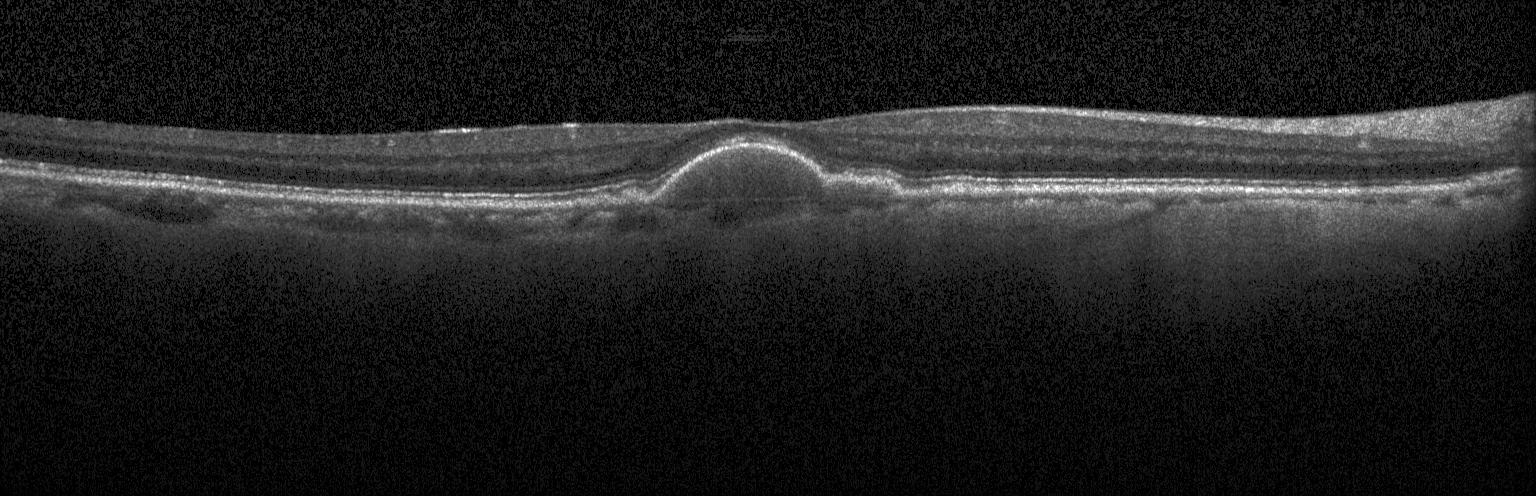

Acquired on a Heidelberg Spectralis; through the macula; spectral-domain optical coherence tomography; retinal OCT cross-section.
Finding: a choroidal neovascular membrane.